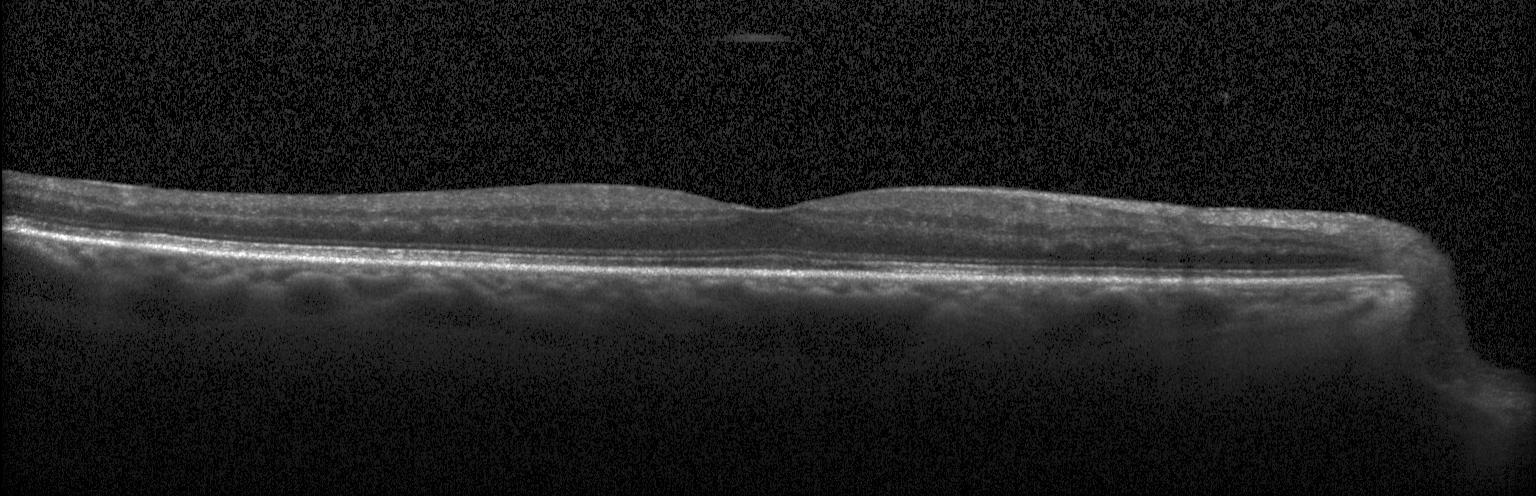

Retinal OCT cross-section. SD-OCT
Finding: neither CNV, DME, nor drusen.